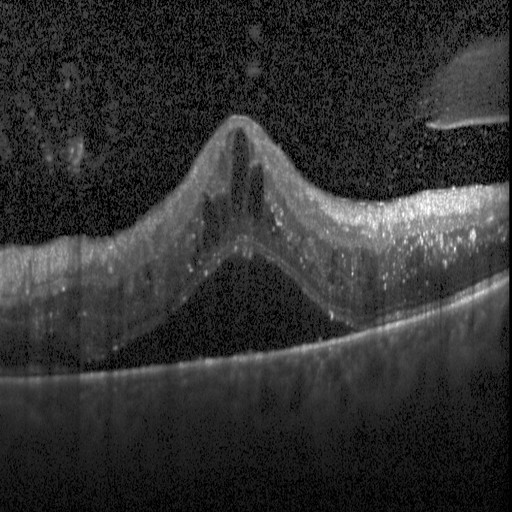 SD-OCT. Retinal OCT B-scan
This B-scan demonstrates DME.